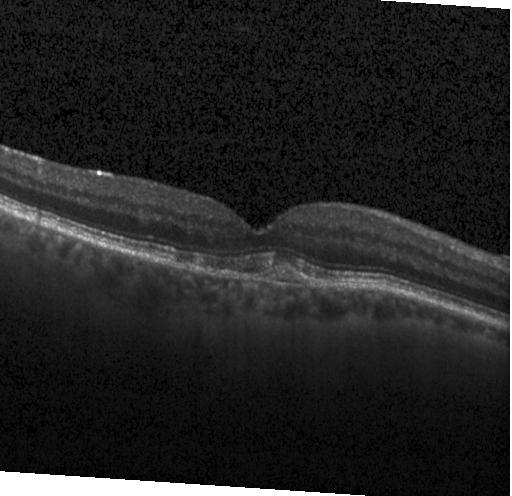
Dx: a choroidal neovascular membrane.